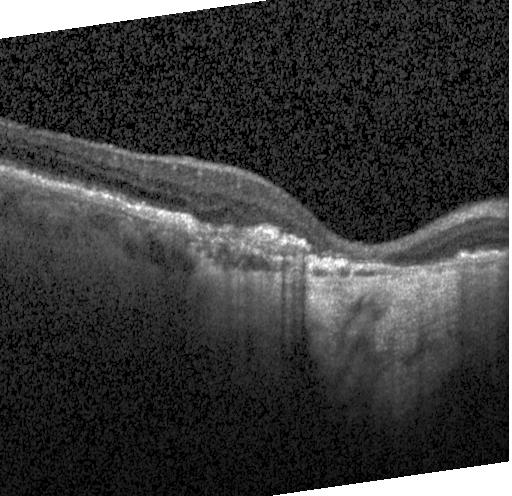 OCT scan showing choroidal neovascularization.